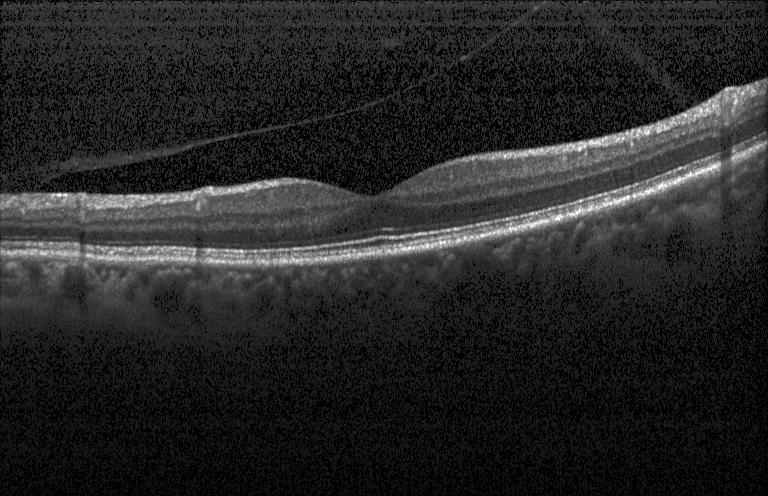

OCT scan showing no choroidal neovascularization, diabetic macular edema, or drusen.